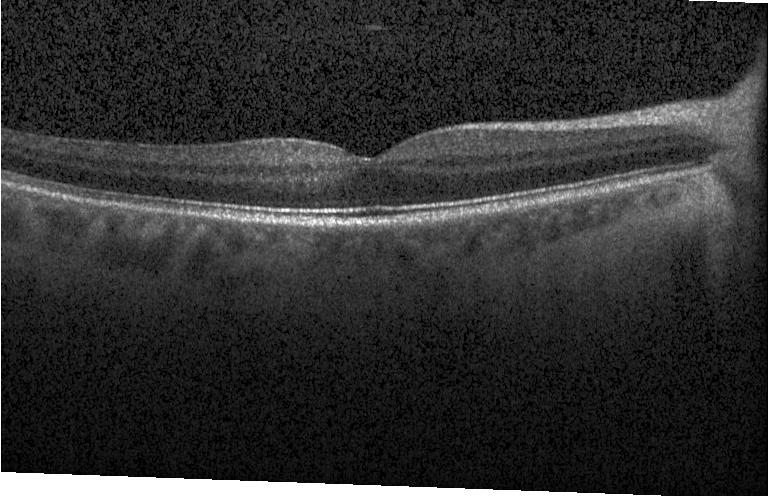
Finding: no choroidal neovascularization, diabetic macular edema, or drusen.